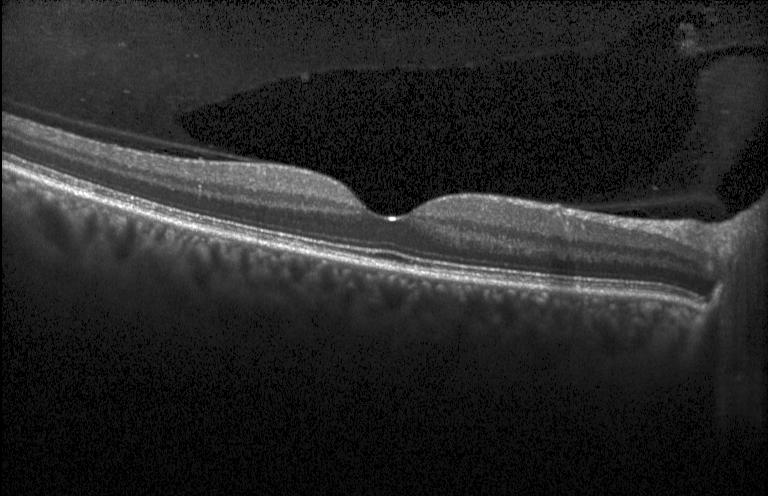
OCT B-scan.
The scan shows no choroidal neovascularization, diabetic macular edema, or drusen.